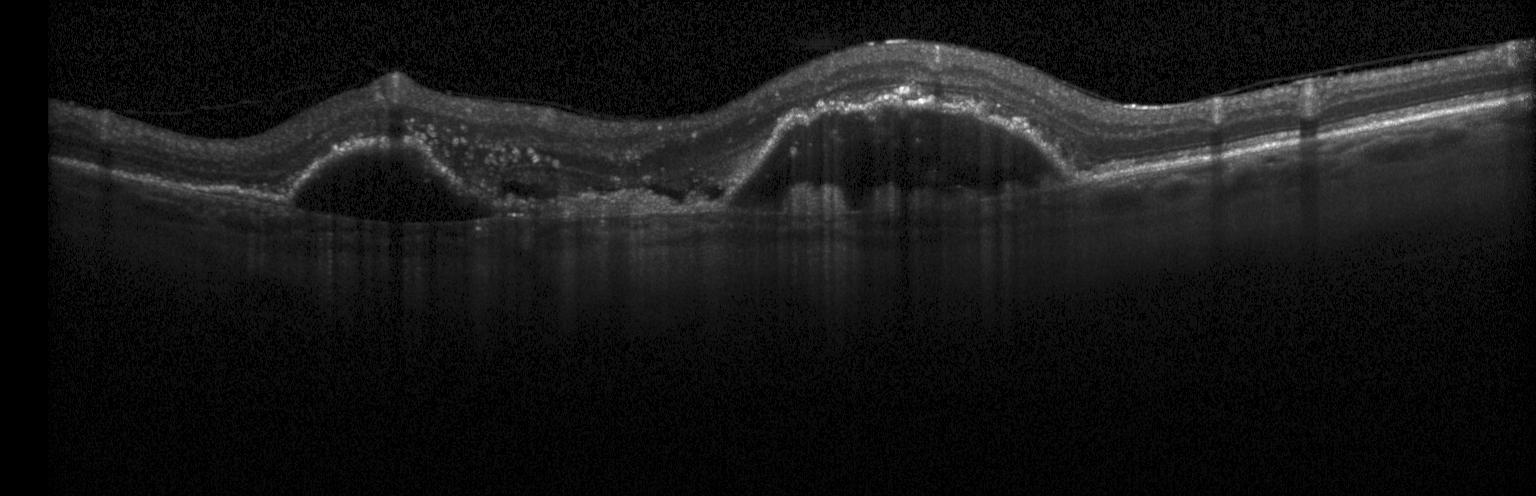
Dx: a choroidal neovascular membrane.